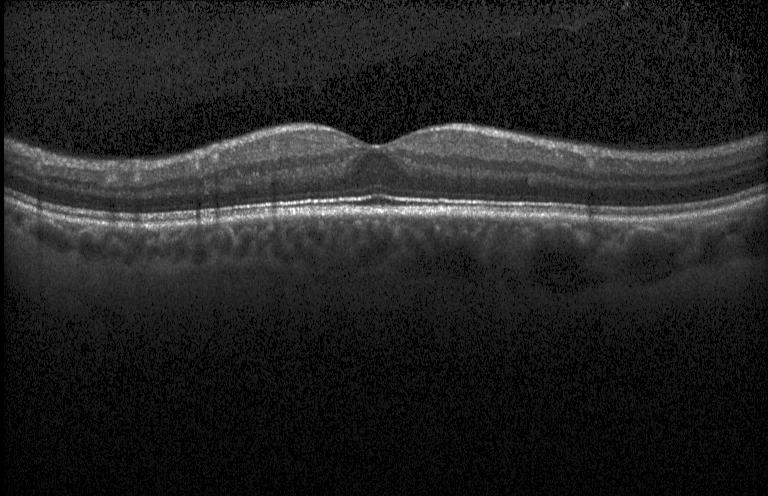
Macular scan · OCT B-scan
Assessment: neither CNV, DME, nor drusen.